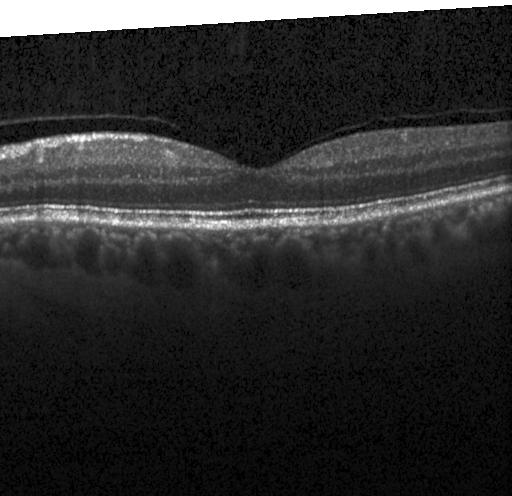

Acquired on a Heidelberg Spectralis; spectral-domain optical coherence tomography; retinal OCT cross-section.
Diagnosis: neither choroidal neovascularization, diabetic macular edema, nor drusen.